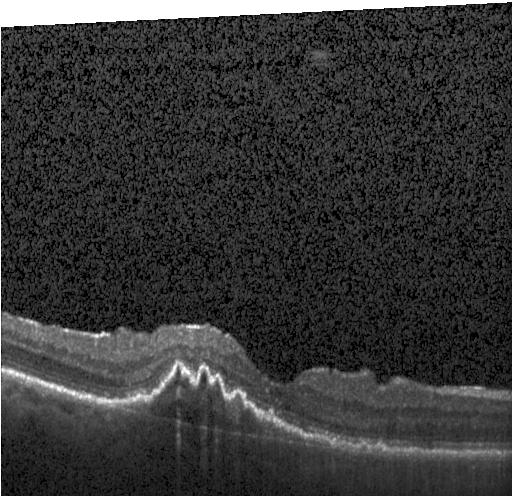 A choroidal neovascular membrane.